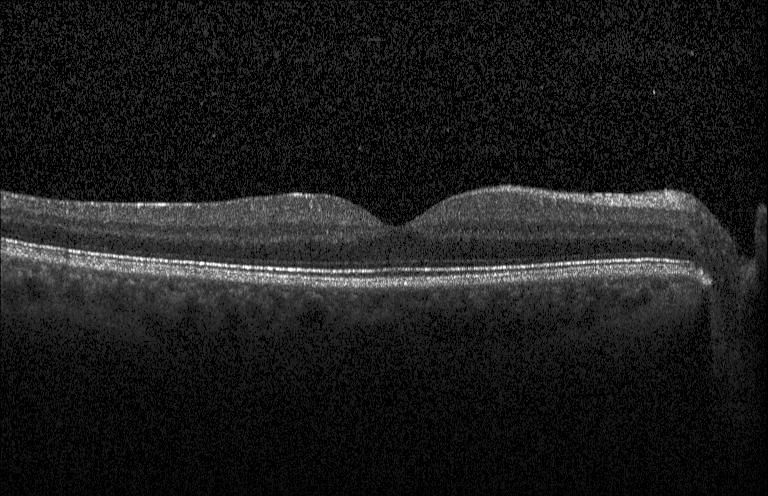

Optical coherence tomography scan. Impression: no choroidal neovascularization, no diabetic macular edema, and no drusen.